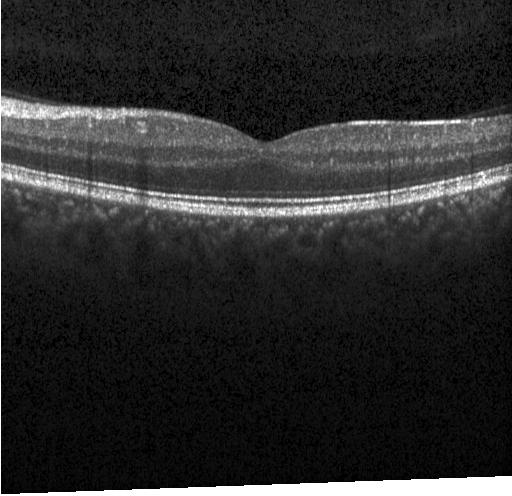 Heidelberg Spectralis. Macular scan. SD-OCT. OCT line scan — Macular OCT: neither choroidal neovascularization, diabetic macular edema, nor drusen.